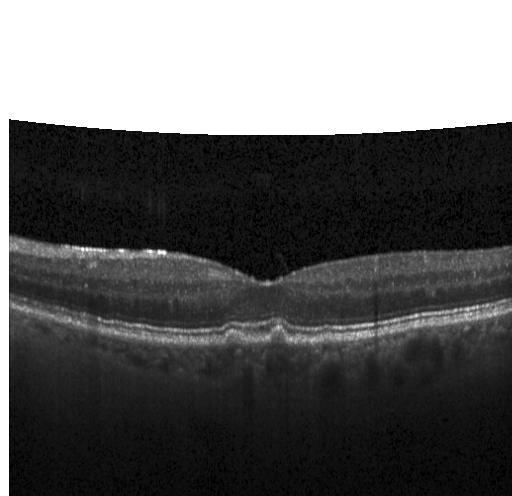
OCT B-scan, SD-OCT.
This B-scan demonstrates drusen.